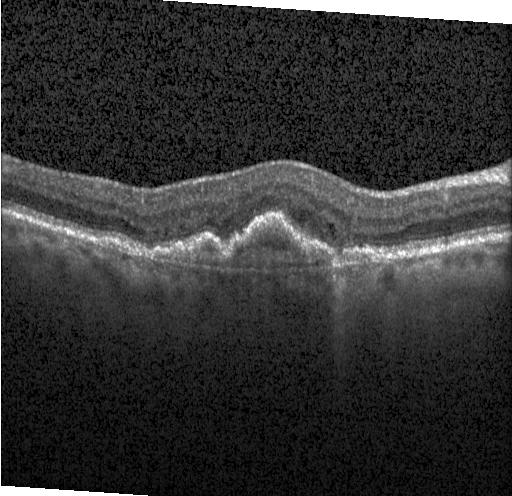 OCT finding: choroidal neovascularization (CNV).